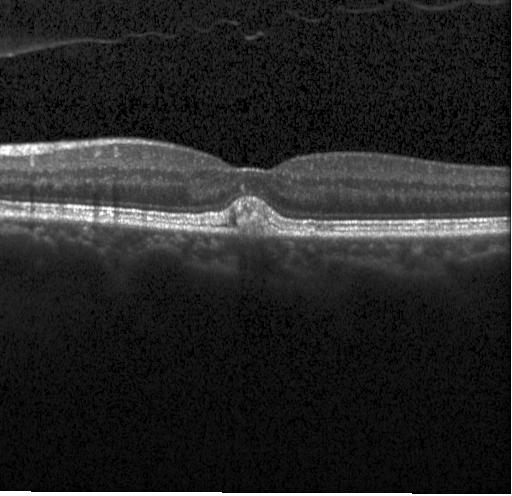
OCT B-scan
Impression: sub-RPE drusenoid deposits.